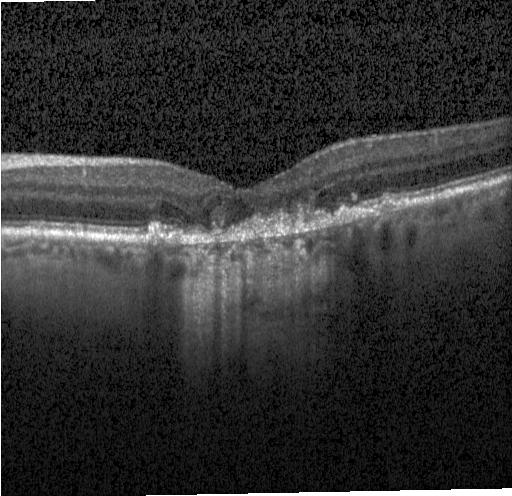 Spectral-domain optical coherence tomography · horizontal scan through the fovea · instrument: Heidelberg Spectralis · OCT line scan. Impression: a choroidal neovascular membrane.